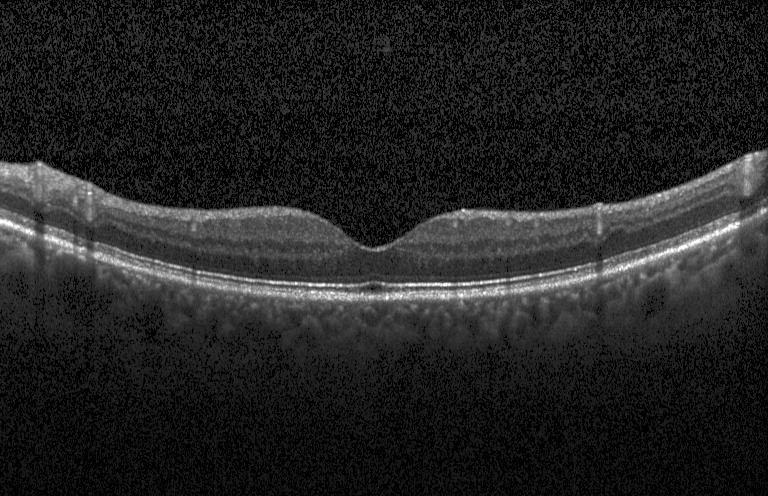

OCT B-scan.
This B-scan demonstrates no choroidal neovascularization, diabetic macular edema, or drusen.